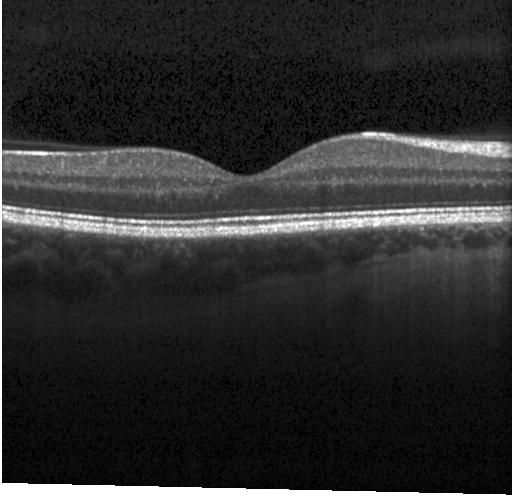 OCT line scan.
The scan shows no choroidal neovascularization, diabetic macular edema, or drusen.